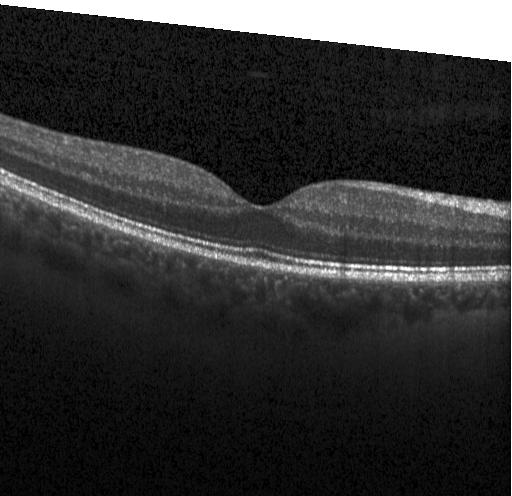 OCT B-scan. SD-OCT. Horizontal scan through the fovea — OCT finding: no evidence of choroidal neovascularization, diabetic macular edema, or drusen.